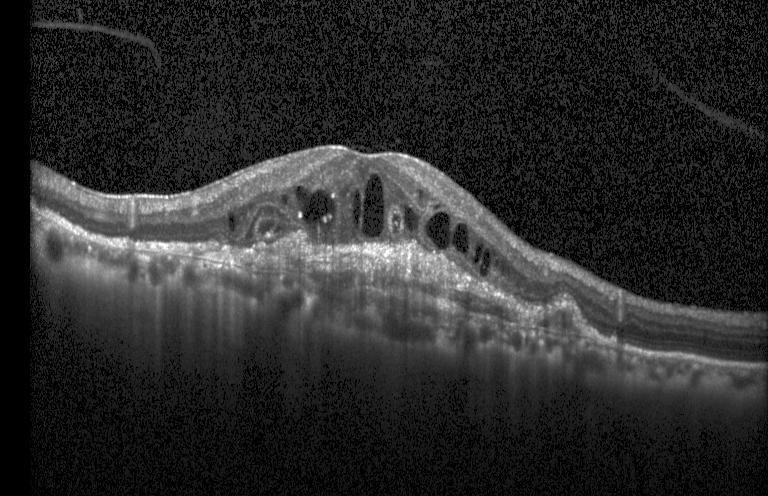
Instrument: Heidelberg Spectralis · fovea-centered · SD-OCT · retinal OCT cross-section. The scan shows a choroidal neovascular membrane.